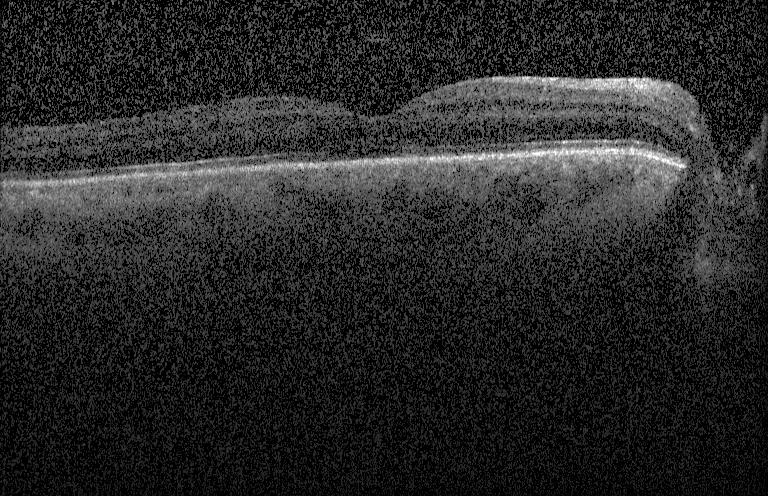
Centered on the fovea. OCT B-scan. Spectral-domain optical coherence tomography
Dx: no choroidal neovascularization, diabetic macular edema, or drusen.